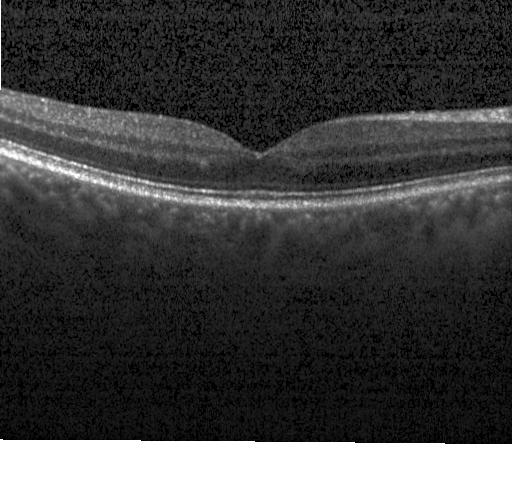 Spectral-domain OCT B-scan: no CNV, DME, or drusen.